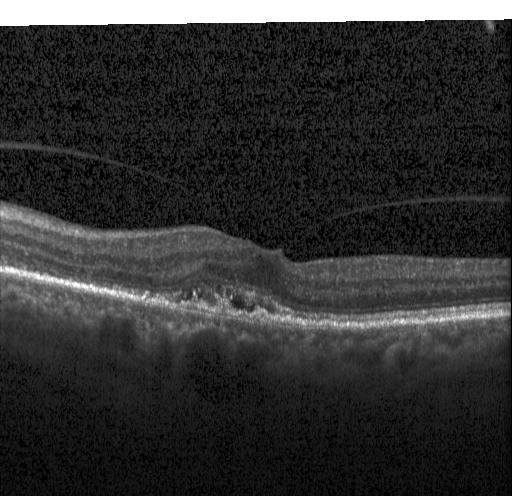

Spectral-domain OCT; acquired on a Heidelberg Spectralis; optical coherence tomography scan
Impression: a choroidal neovascular membrane.